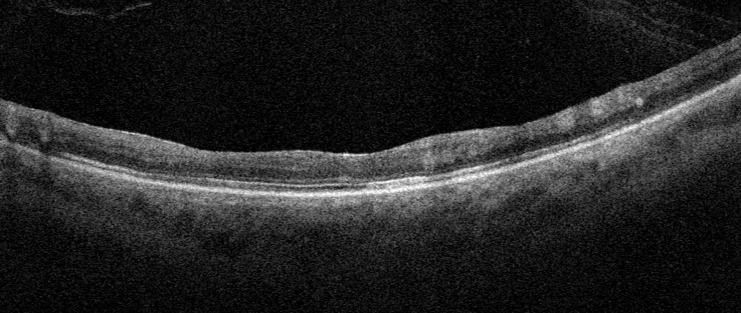 OCT B-scan, instrument: Optovue Avanti RTVue XR, macular scan. OCT finding: age-related macular degeneration (AMD).